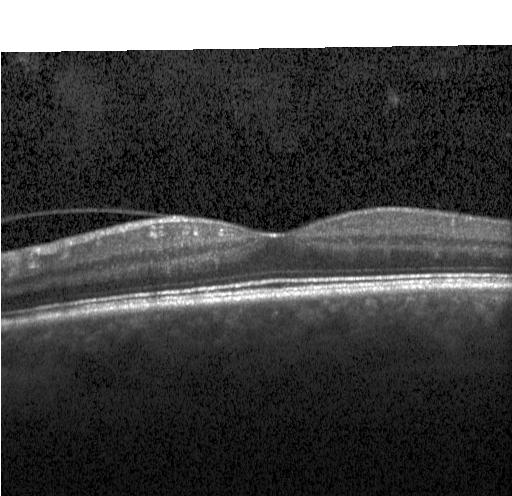

OCT B-scan. Through the macula. Heidelberg Spectralis. Assessment: no CNV, no DME, and no drusen.